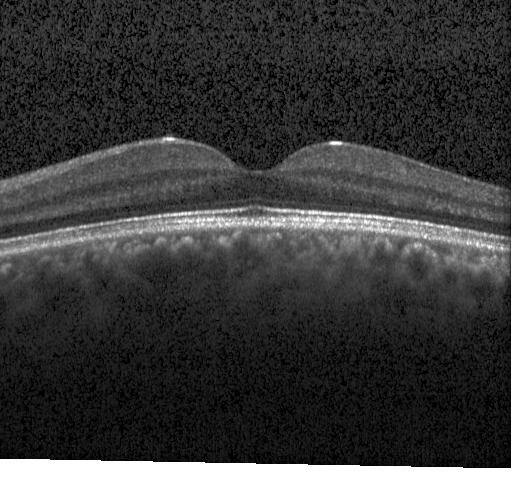

OCT finding: no choroidal neovascularization, no diabetic macular edema, and no drusen.